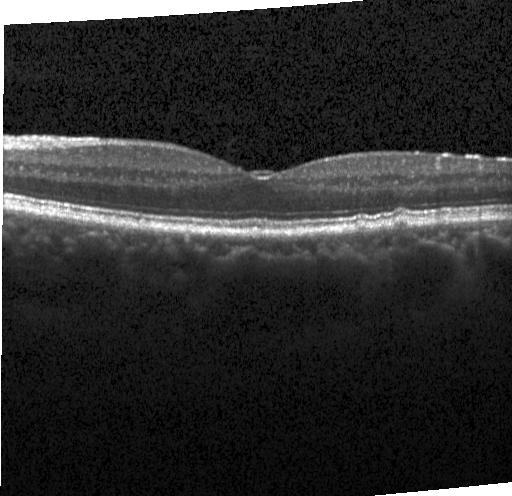

Retinal OCT cross-section, spectral-domain optical coherence tomography
Diagnosis: multiple drusen.